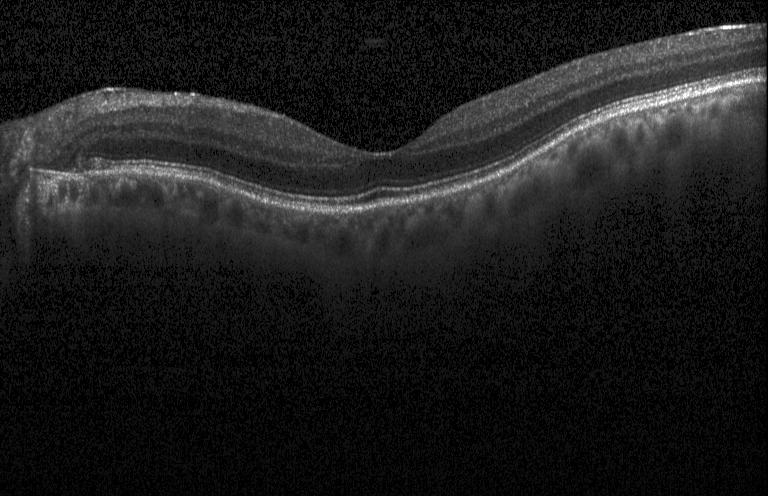 Through the macula; OCT B-scan
OCT finding: neither choroidal neovascularization, diabetic macular edema, nor drusen.